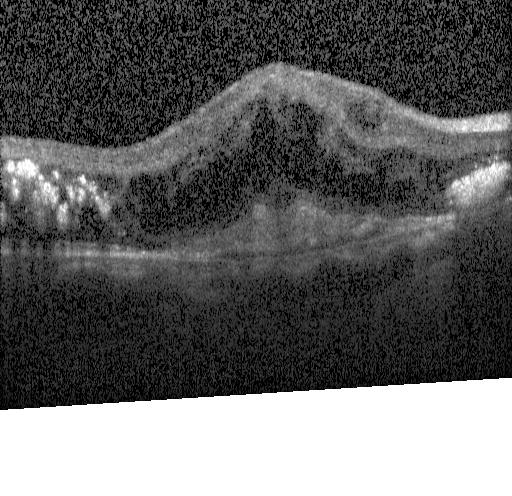 Centered on the fovea, retinal OCT B-scan — Diagnosis: a choroidal neovascular membrane.